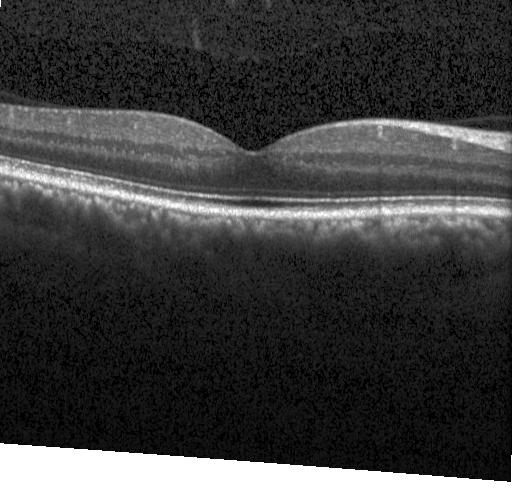 Assessment: no choroidal neovascularization, no diabetic macular edema, and no drusen.